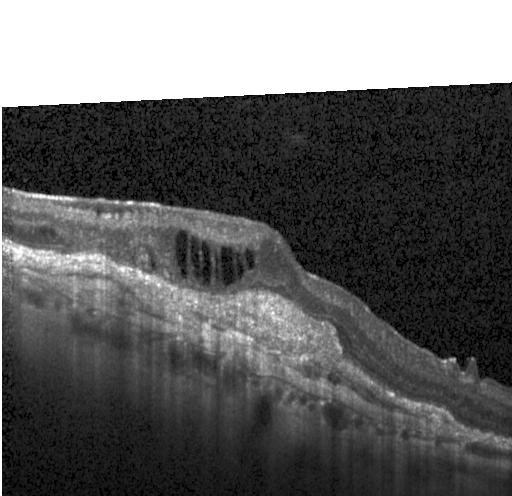
OCT line scan, fovea-centered
Choroidal neovascularization (CNV).